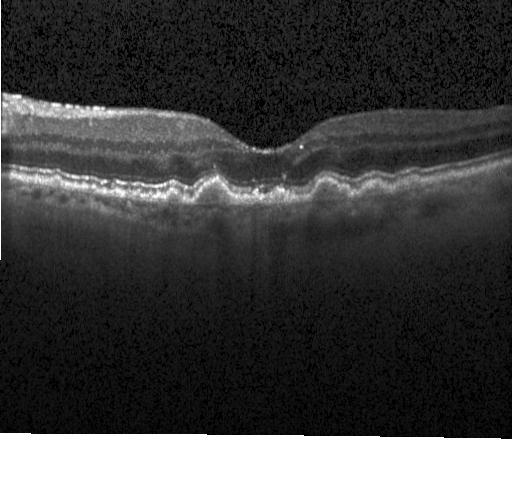

Instrument: Heidelberg Spectralis. OCT B-scan
Macular OCT: multiple drusen.